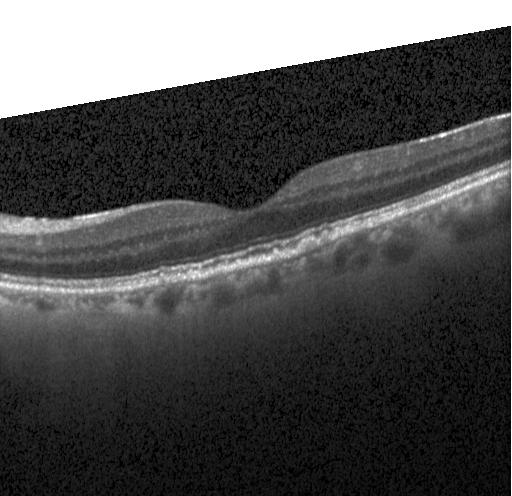

Centered on the fovea · retinal OCT cross-section
Diagnosis: drusen.